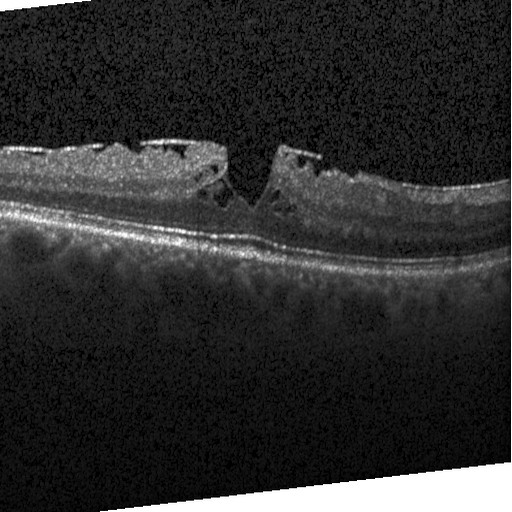 Finding: DME.